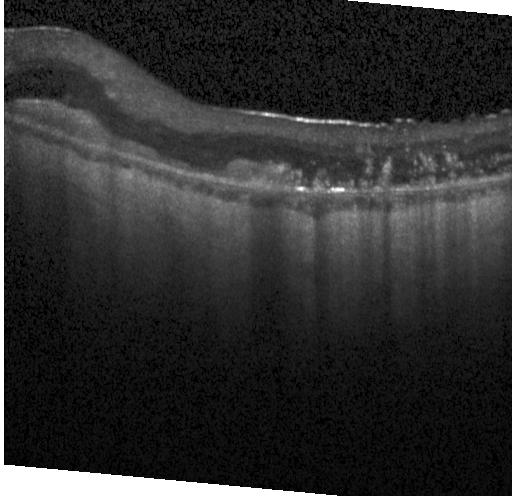
SD-OCT · retinal OCT B-scan · horizontal scan through the fovea · acquired on a Heidelberg Spectralis.
Diagnosis: a choroidal neovascular membrane.